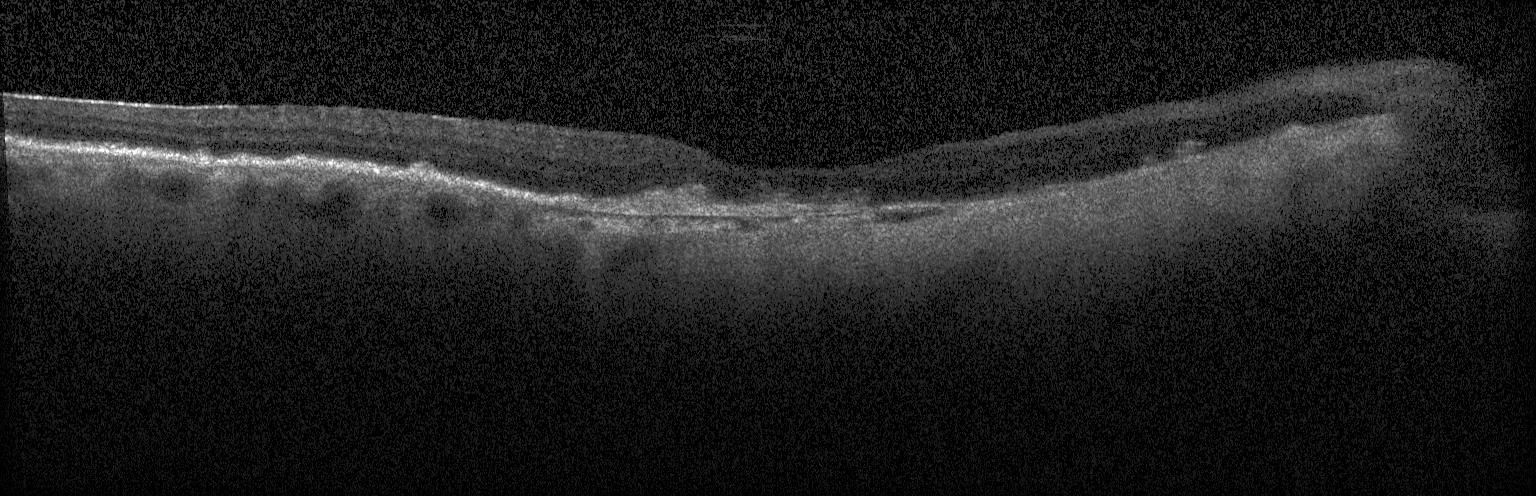
OCT scan showing CNV.